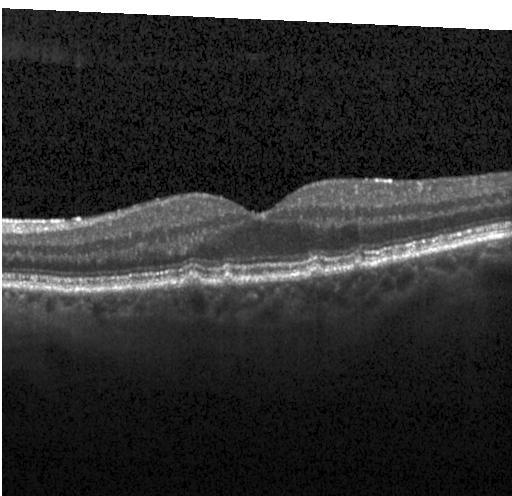 Diagnosis: drusen.